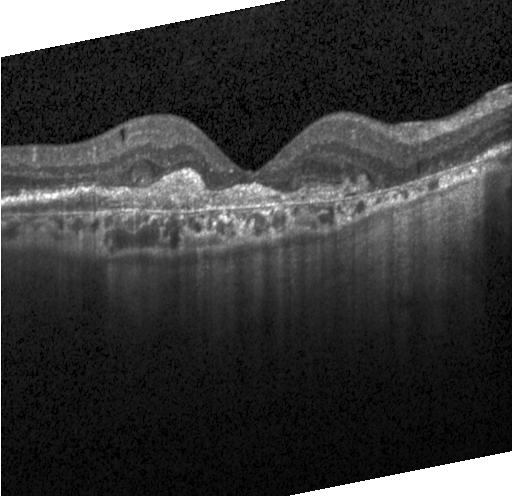

Heidelberg Spectralis, centered on the fovea, retinal OCT cross-section, SD-OCT.
This B-scan demonstrates CNV.